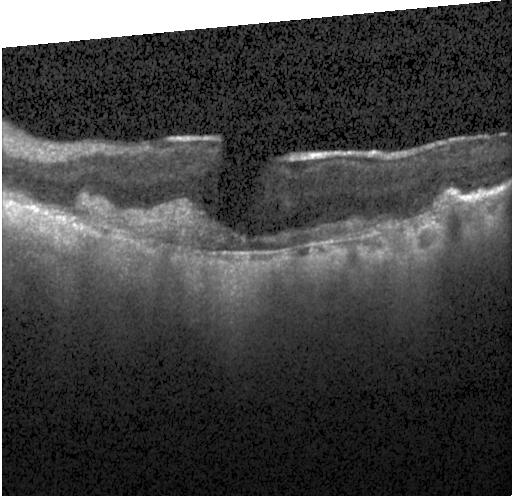
This B-scan demonstrates choroidal neovascularization.